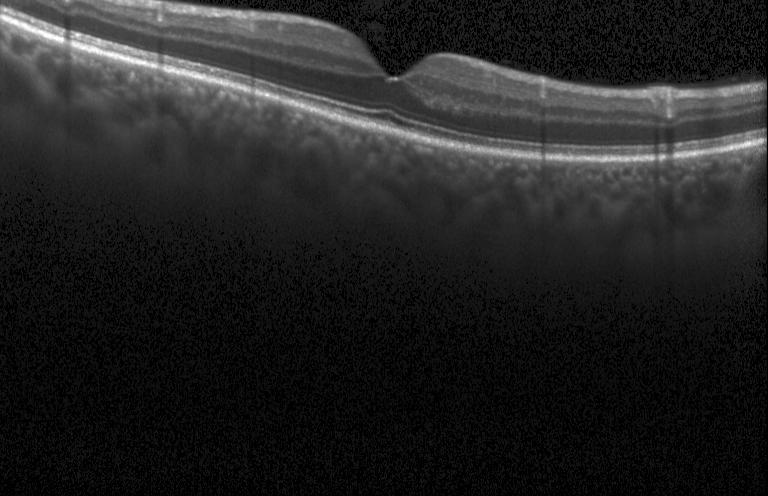

Spectral-domain optical coherence tomography, OCT line scan
No evidence of choroidal neovascularization, diabetic macular edema, or drusen.